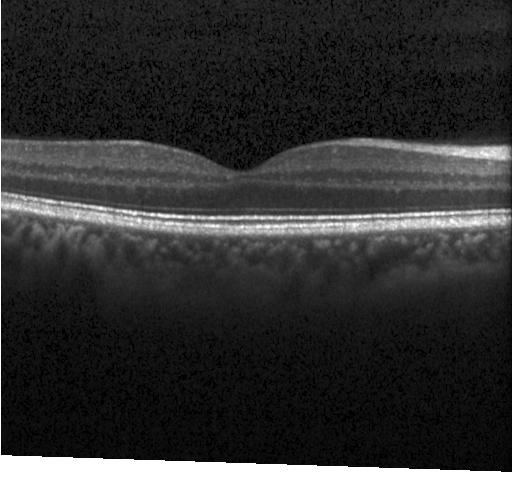 Spectral-domain optical coherence tomography · OCT B-scan · Heidelberg Spectralis OCT system · centered on the fovea.
Finding: no CNV, DME, or drusen.